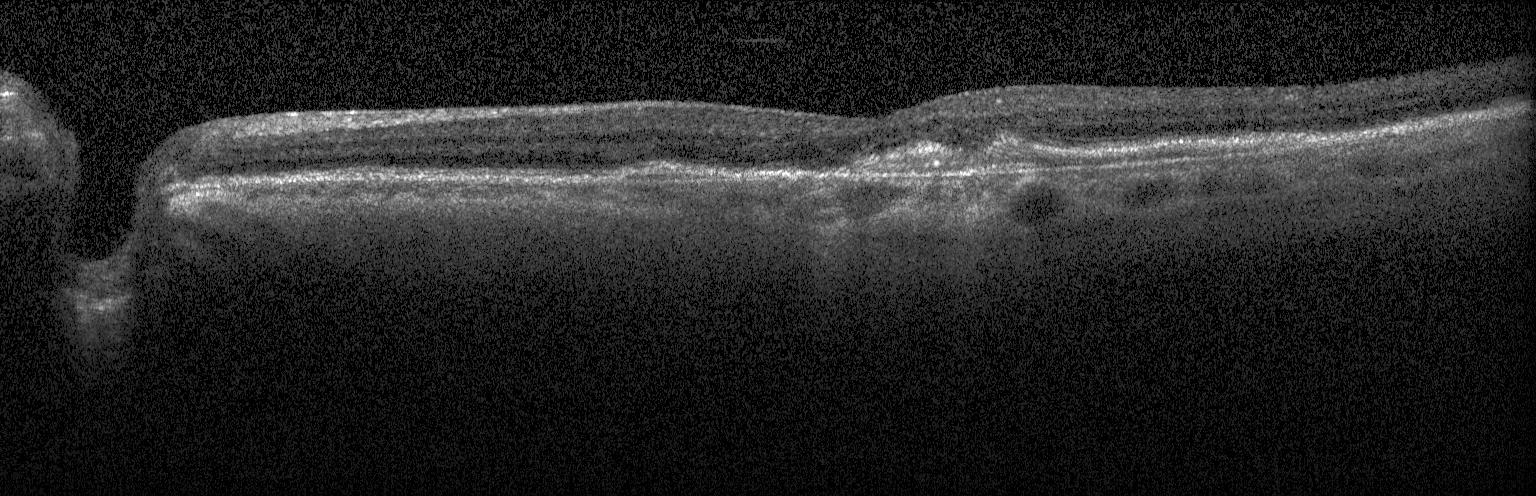
Impression: a choroidal neovascular membrane.